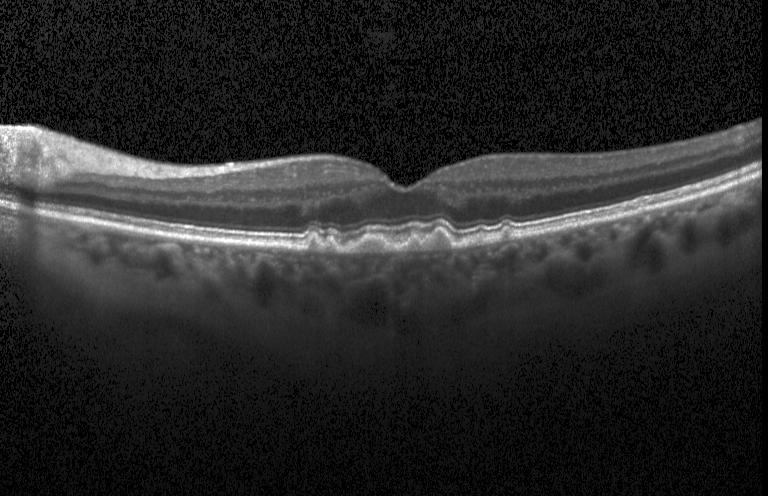

Heidelberg Spectralis, OCT B-scan — Impression: multiple drusen.